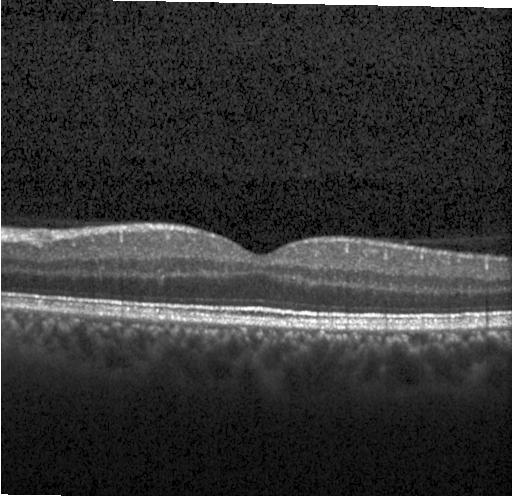

Retinal OCT B-scan · Heidelberg Spectralis OCT system · macular scan. Neither choroidal neovascularization, diabetic macular edema, nor drusen.